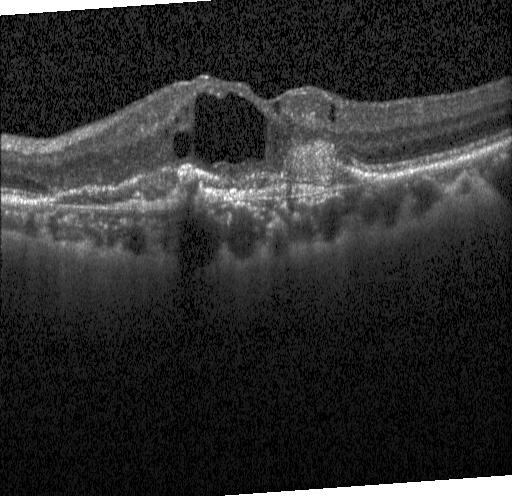

Centered on the fovea; optical coherence tomography scan; spectral-domain optical coherence tomography; instrument: Heidelberg Spectralis — Finding: CNV.